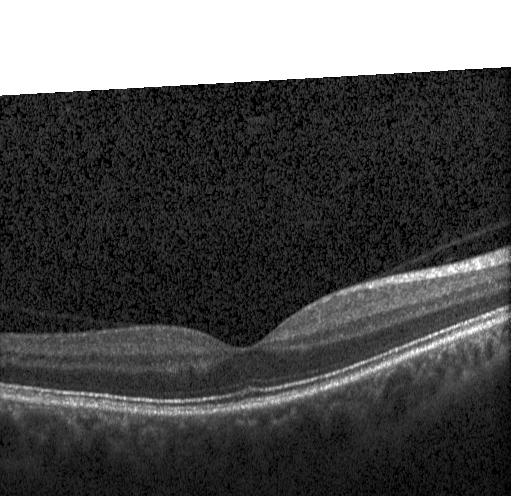 Acquired on a Heidelberg Spectralis; fovea-centered; spectral-domain optical coherence tomography; OCT B-scan — Neither choroidal neovascularization, diabetic macular edema, nor drusen.